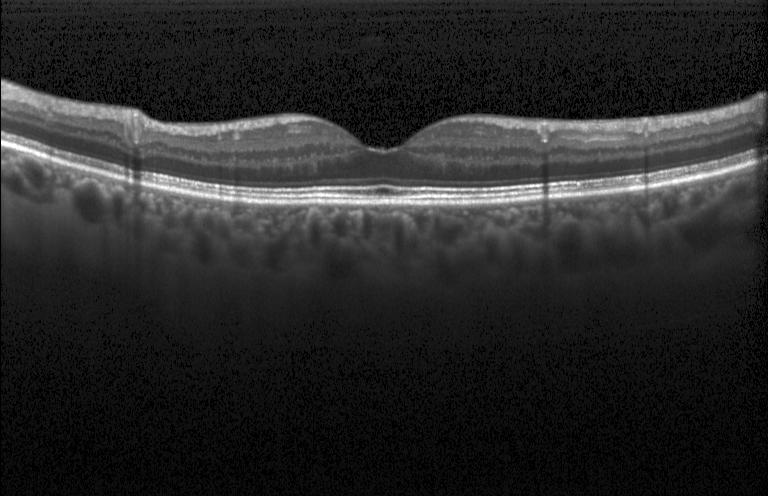

Heidelberg Spectralis OCT system; optical coherence tomography B-scan; macular scan; spectral-domain OCT.
Macular OCT: no evidence of choroidal neovascularization, diabetic macular edema, or drusen.